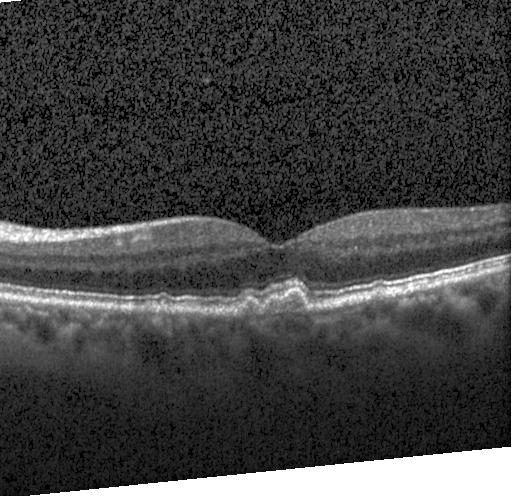

Macular OCT: sub-RPE drusenoid deposits.